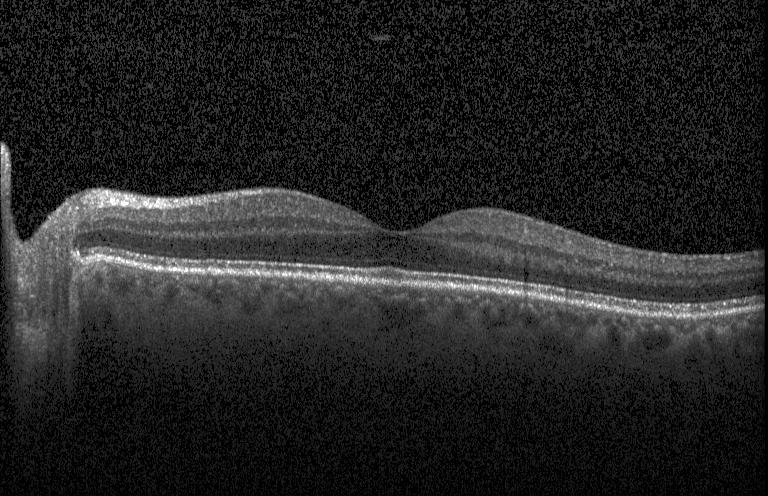

Spectral-domain OCT; centered on the fovea; Heidelberg Spectralis; retinal OCT cross-section.
Diagnosis: no choroidal neovascularization, diabetic macular edema, or drusen.